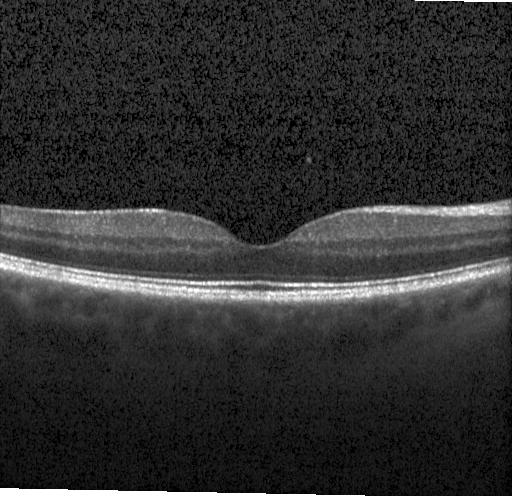

Optical coherence tomography scan.
No choroidal neovascularization, diabetic macular edema, or drusen.